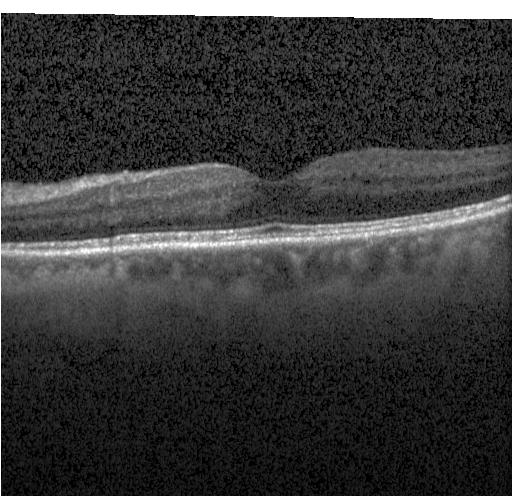
OCT B-scan showing neither choroidal neovascularization, diabetic macular edema, nor drusen.